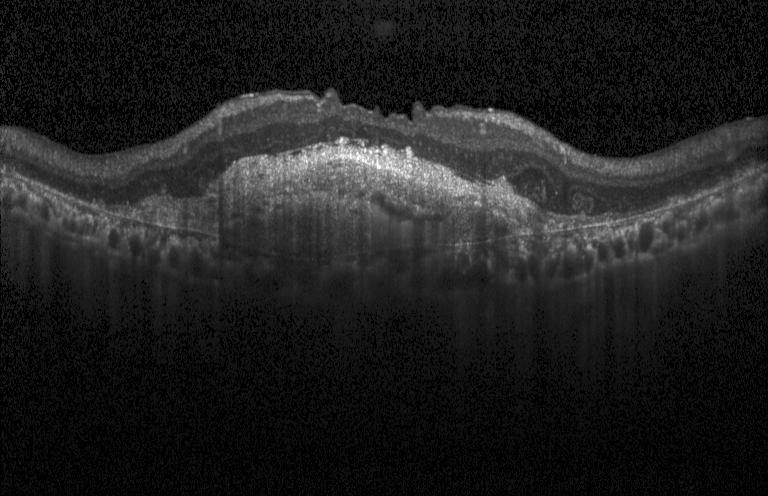 Macular OCT demonstrating a choroidal neovascular membrane.